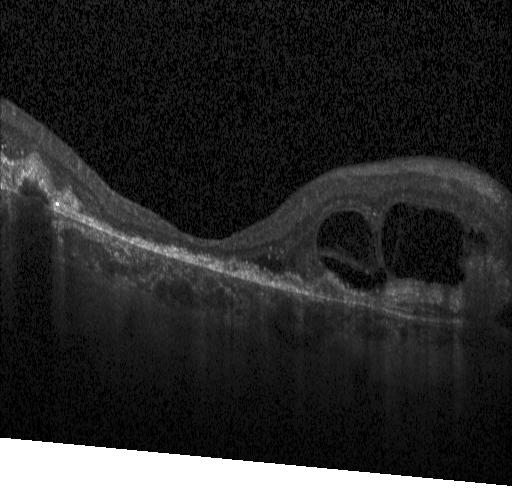

SD-OCT, OCT line scan, instrument: Heidelberg Spectralis, horizontal scan through the fovea. Dx: choroidal neovascularization.